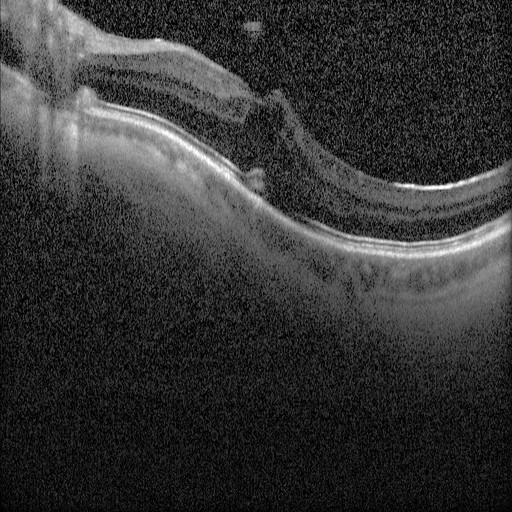 OCT B-scan; SD-OCT; horizontal scan through the fovea. OCT finding: DME.